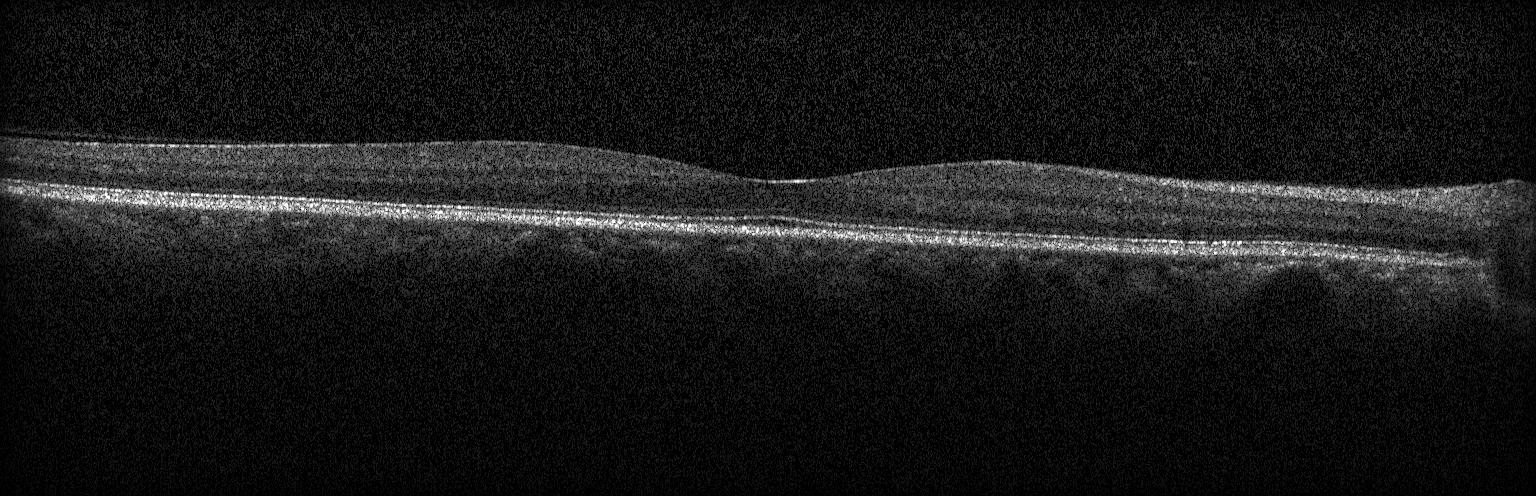
Centered on the fovea; optical coherence tomography B-scan; spectral-domain optical coherence tomography.
Impression: no evidence of choroidal neovascularization, diabetic macular edema, or drusen.